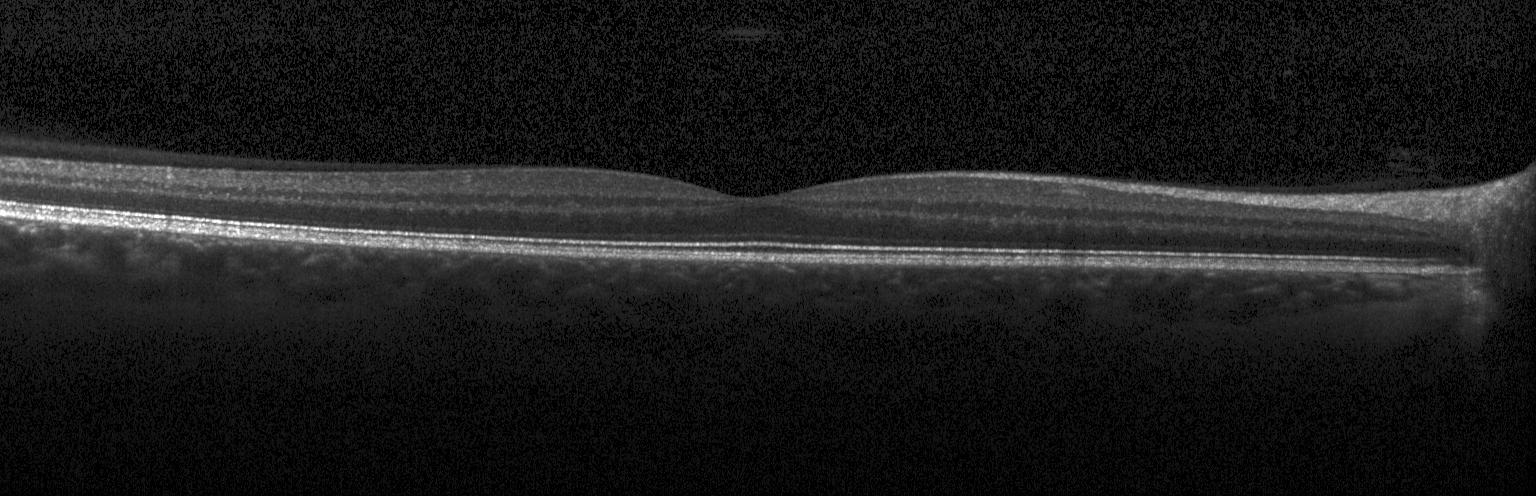 Retinal OCT B-scan
Assessment: no CNV, DME, or drusen.